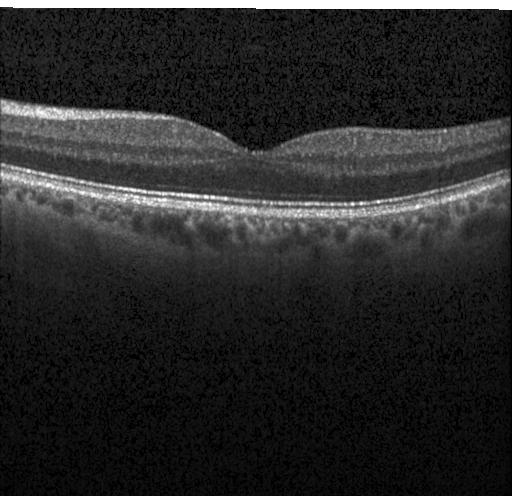

Impression: no CNV, no DME, and no drusen.